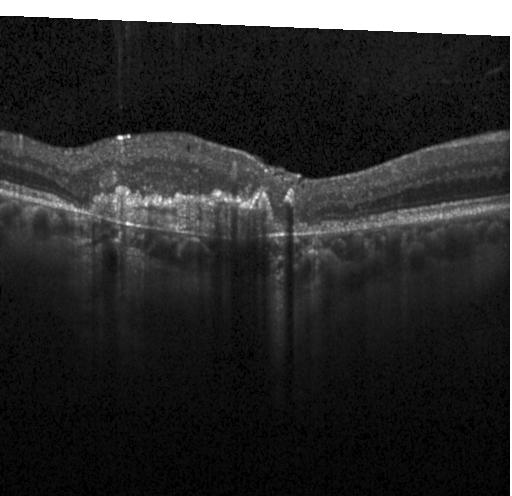
Optical coherence tomography B-scan. SD-OCT
The scan shows CNV.